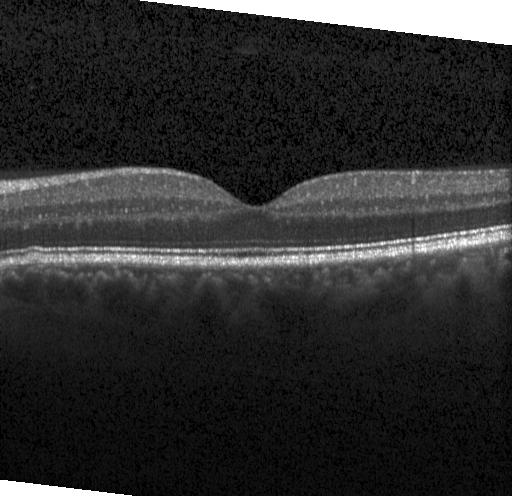
SD-OCT, optical coherence tomography B-scan.
No evidence of choroidal neovascularization, diabetic macular edema, or drusen.